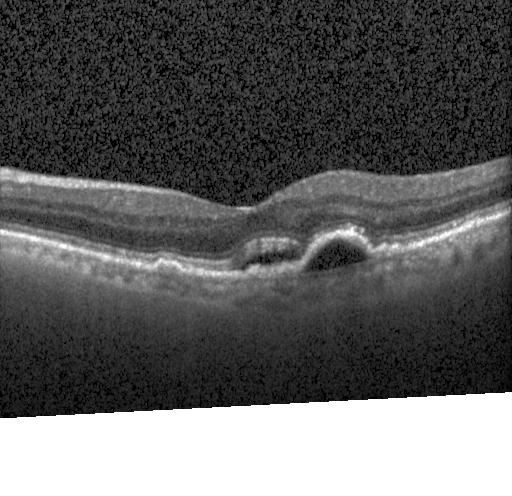

Spectral-domain OCT · retinal OCT cross-section · acquired on a Heidelberg Spectralis · centered on the fovea — Macular OCT: a choroidal neovascular membrane.